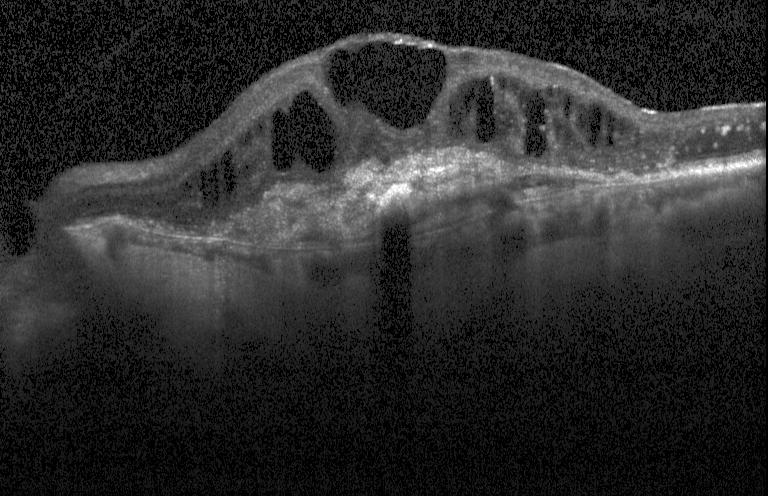

Diagnosis: a choroidal neovascular membrane.